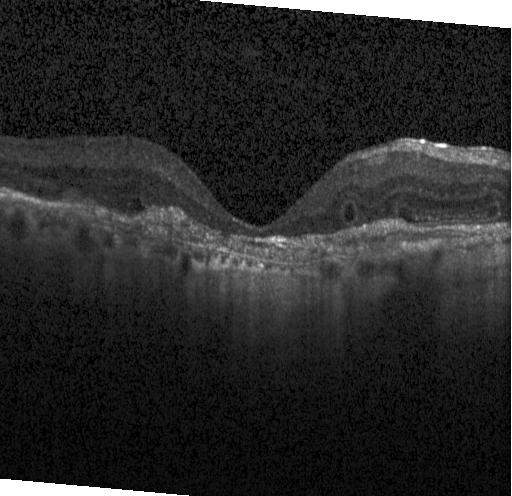
Spectral-domain OCT B-scan: CNV.